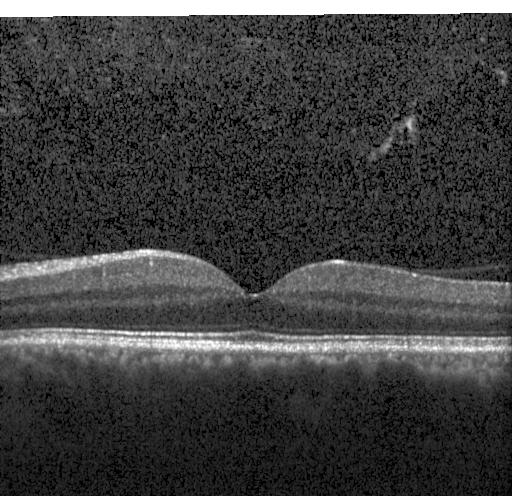
Spectral-domain optical coherence tomography, instrument: Heidelberg Spectralis, optical coherence tomography scan.
Diagnosis: no CNV, DME, or drusen.